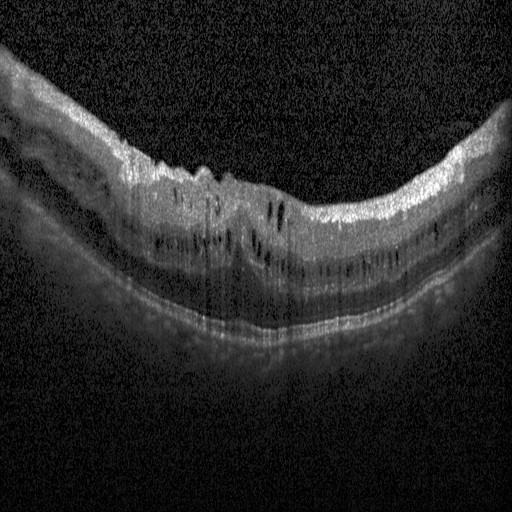
Impression: DME.